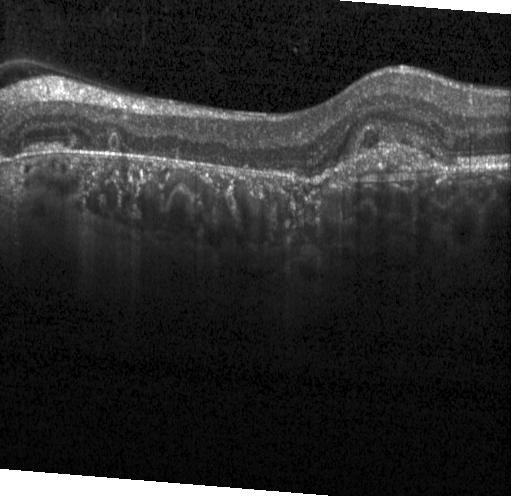

OCT B-scan. Impression: a choroidal neovascular membrane.